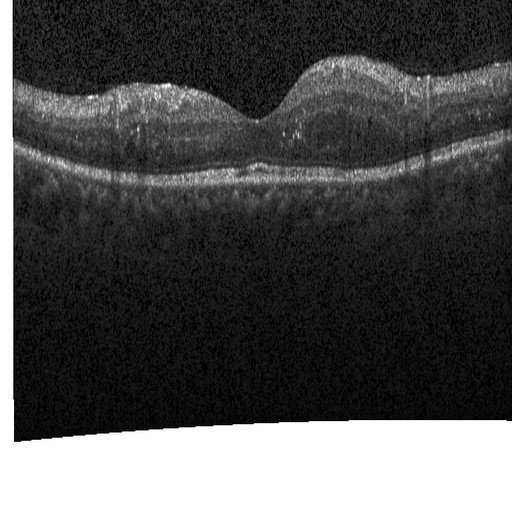

Retinal OCT cross-section, acquired on a Heidelberg Spectralis, macular scan.
Finding: diabetic macular edema (DME).